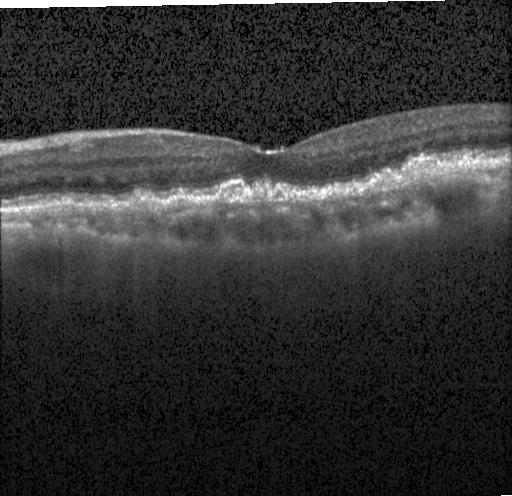 Diagnosis: multiple drusen.